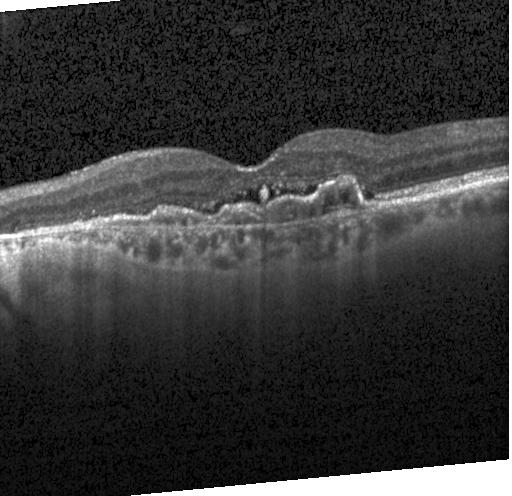 Acquired on a Heidelberg Spectralis. Fovea-centered. Retinal OCT cross-section. Choroidal neovascularization (CNV).